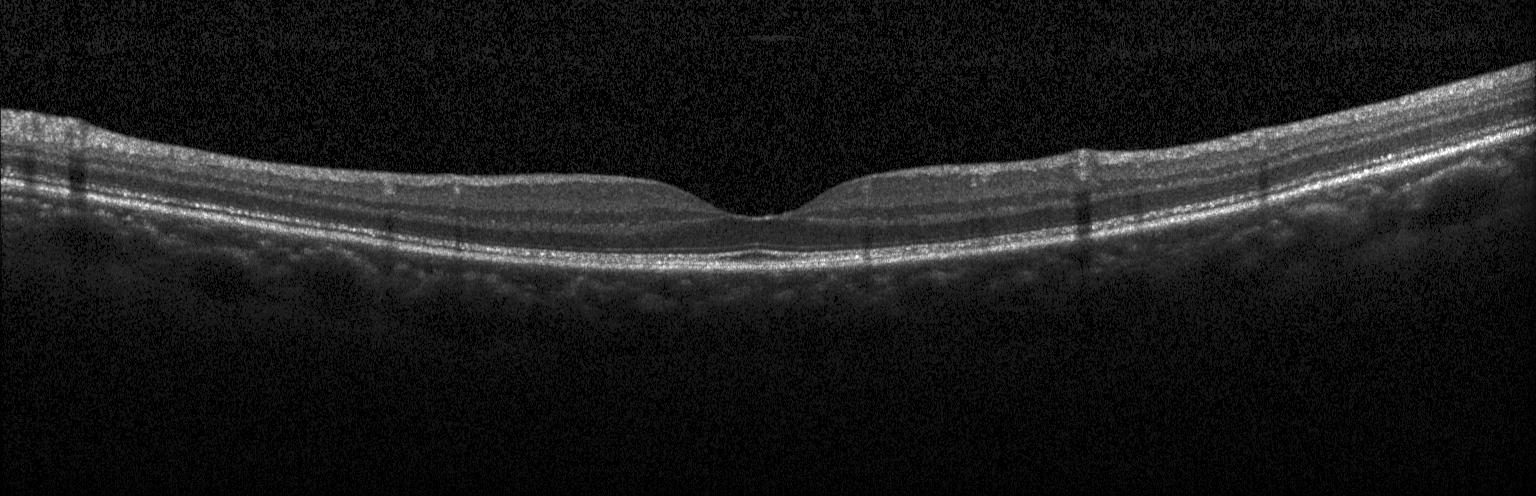 Heidelberg Spectralis, spectral-domain optical coherence tomography, retinal OCT cross-section, centered on the fovea
The scan shows no evidence of choroidal neovascularization, diabetic macular edema, or drusen.